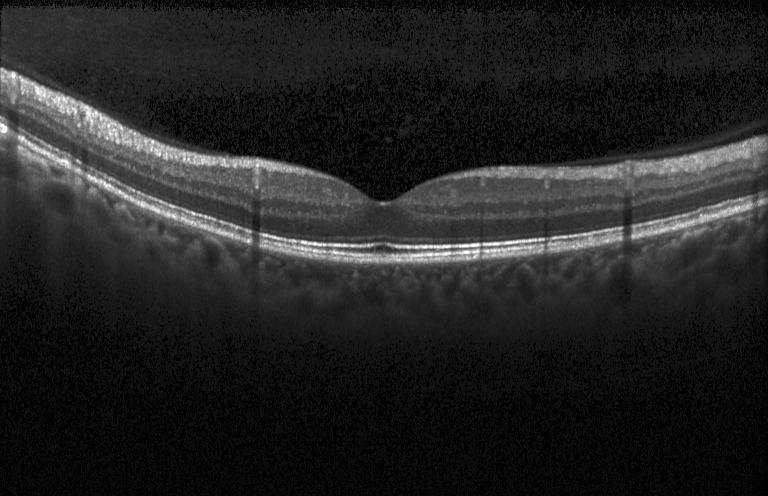

Spectral-domain OCT. Optical coherence tomography B-scan. Fovea-centered. Instrument: Heidelberg Spectralis
Assessment: no choroidal neovascularization, no diabetic macular edema, and no drusen.